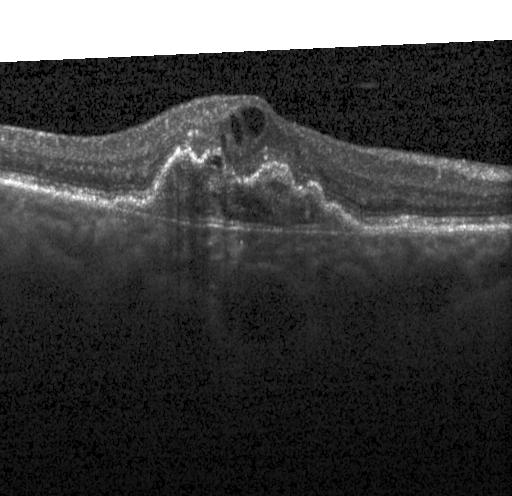 Horizontal scan through the fovea. Spectral-domain optical coherence tomography. Heidelberg Spectralis OCT system. Optical coherence tomography B-scan
Impression: choroidal neovascularization.